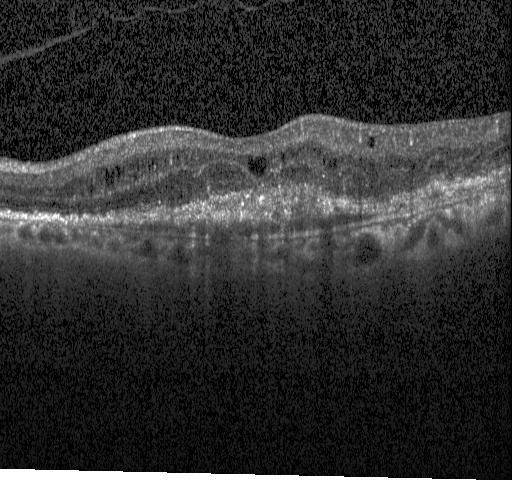 OCT line scan.
Dx: a choroidal neovascular membrane.